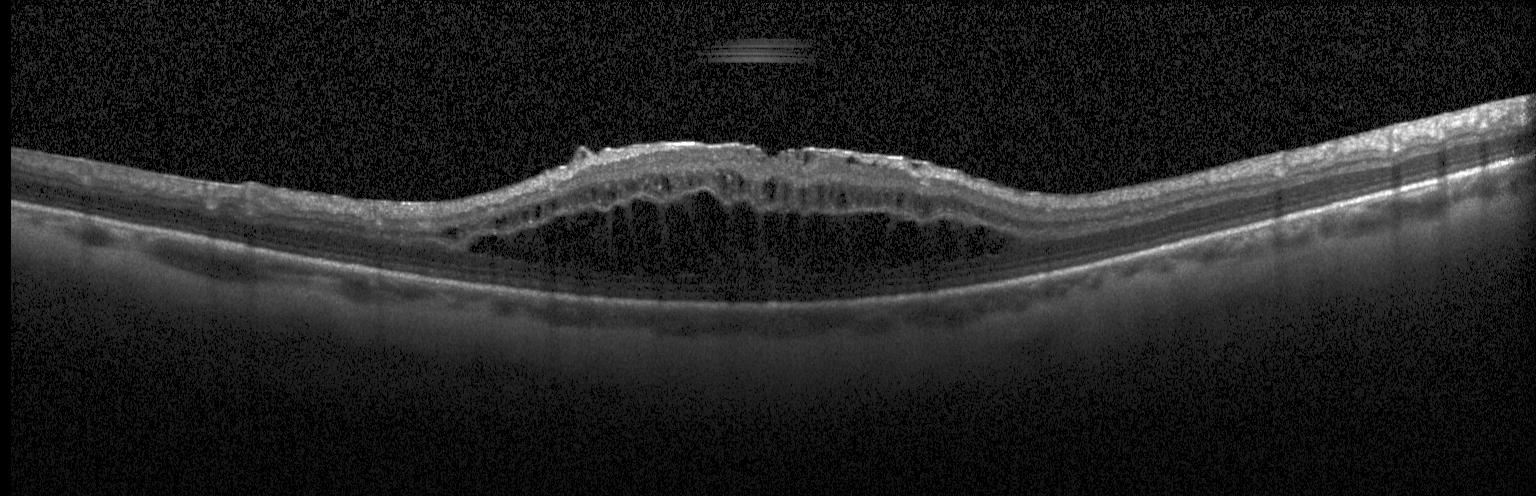 Macular OCT: diabetic macular edema.